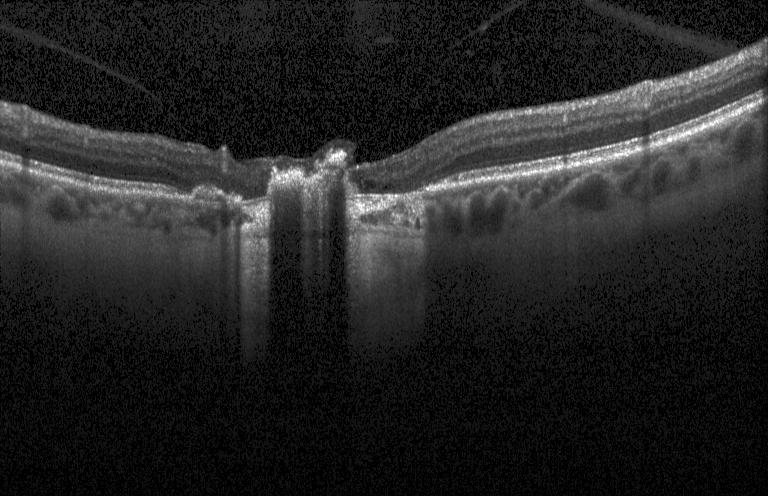
Optical coherence tomography scan.
Finding: a choroidal neovascular membrane.